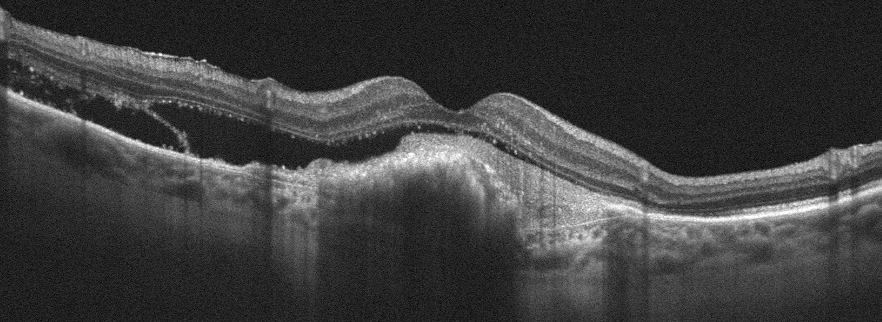
Instrument: Optovue Avanti RTVue XR, fovea-centered, OCT line scan. The scan shows age-related macular degeneration (AMD).